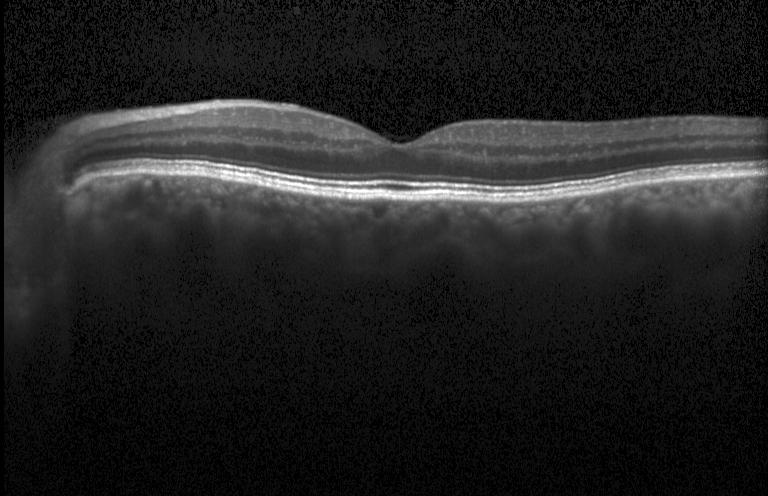 Optical coherence tomography scan
Neither CNV, DME, nor drusen.